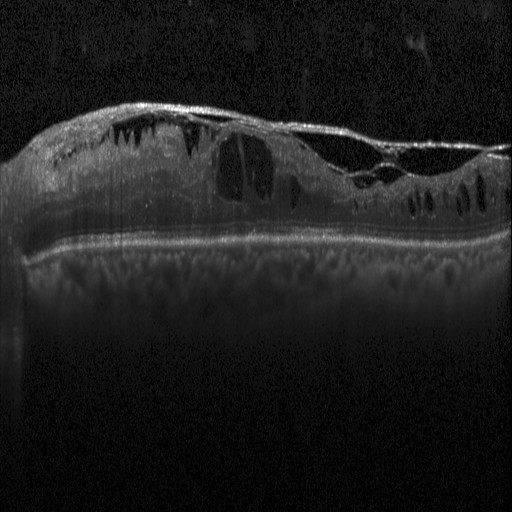

Impression: DME.